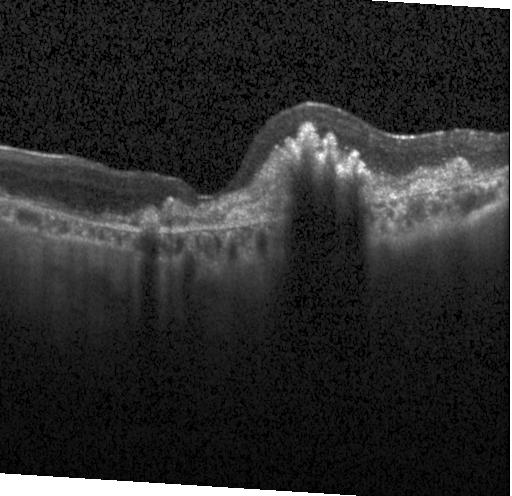
Spectral-domain OCT. Fovea-centered. Retinal OCT cross-section. Diagnosis: a choroidal neovascular membrane.